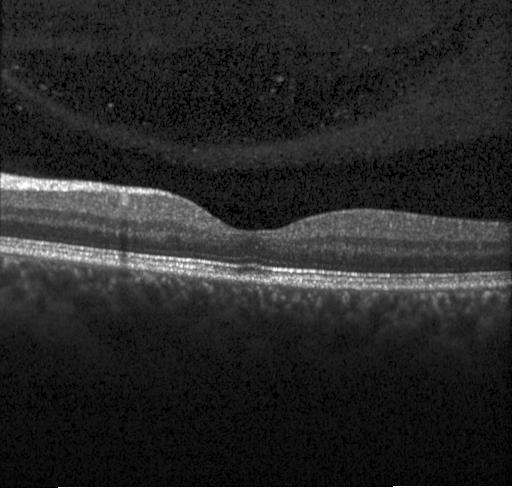

Retinal OCT cross-section
Assessment: no choroidal neovascularization, diabetic macular edema, or drusen.